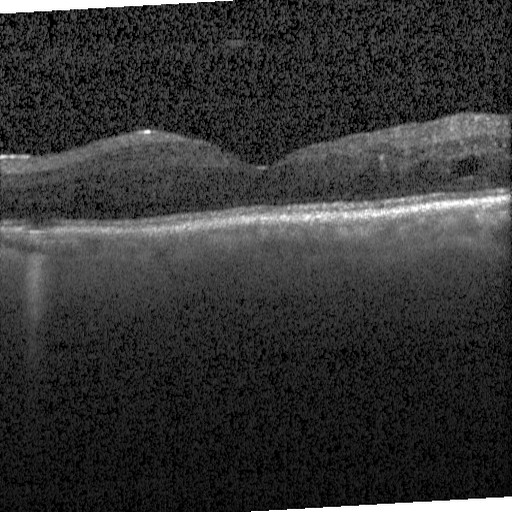 Heidelberg Spectralis OCT system, retinal OCT cross-section, fovea-centered, SD-OCT.
Diagnosis: diabetic macular edema (DME).